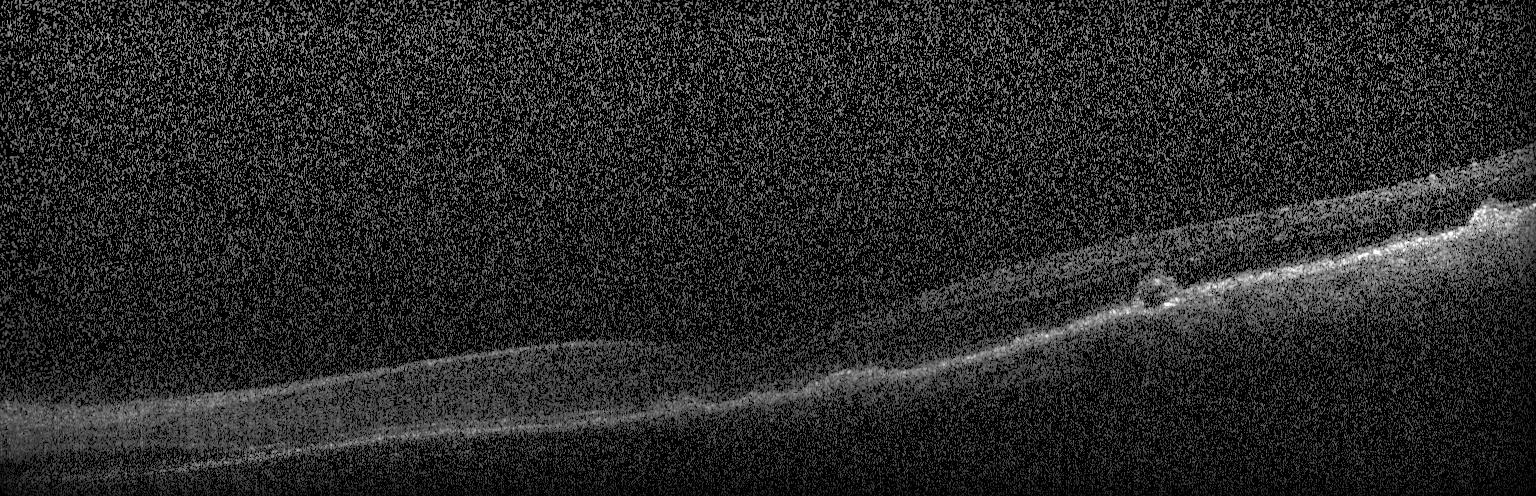 Diagnosis: a choroidal neovascular membrane.